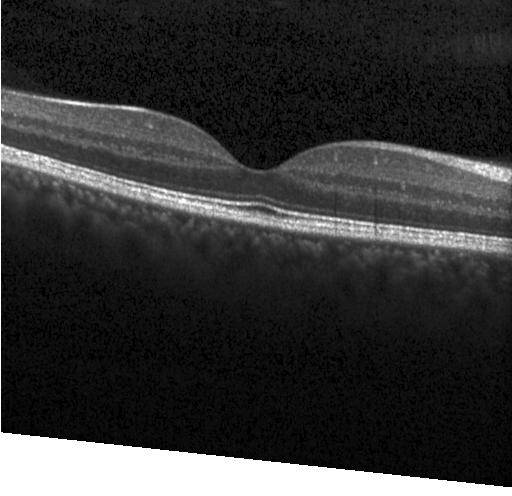
Dx: neither choroidal neovascularization, diabetic macular edema, nor drusen.